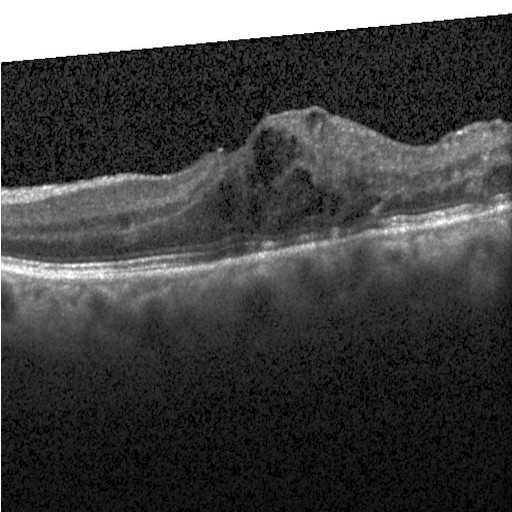

Centered on the fovea. Spectral-domain optical coherence tomography. OCT B-scan. Heidelberg Spectralis — Macular OCT: diabetic macular edema.